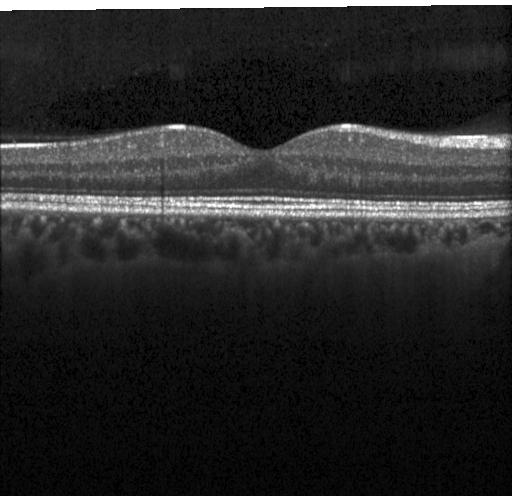 Heidelberg Spectralis OCT system, through the macula, spectral-domain OCT, OCT line scan. Finding: no choroidal neovascularization, no diabetic macular edema, and no drusen.